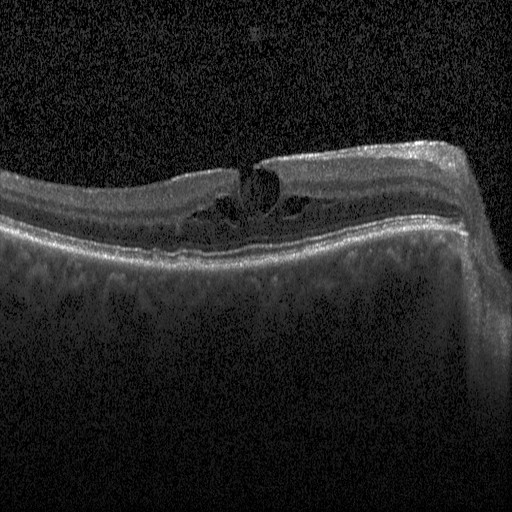 OCT scan showing diabetic macular edema (DME).